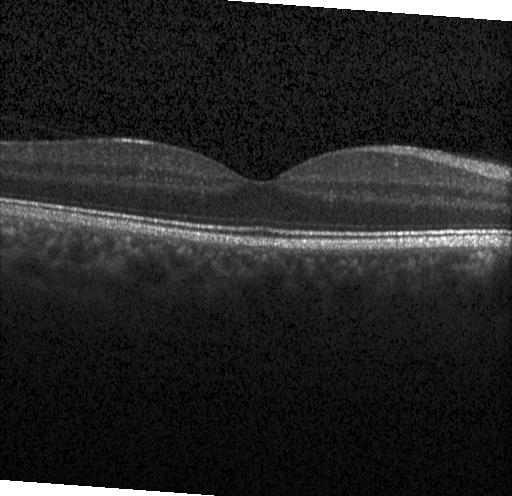
OCT finding: no choroidal neovascularization, diabetic macular edema, or drusen.